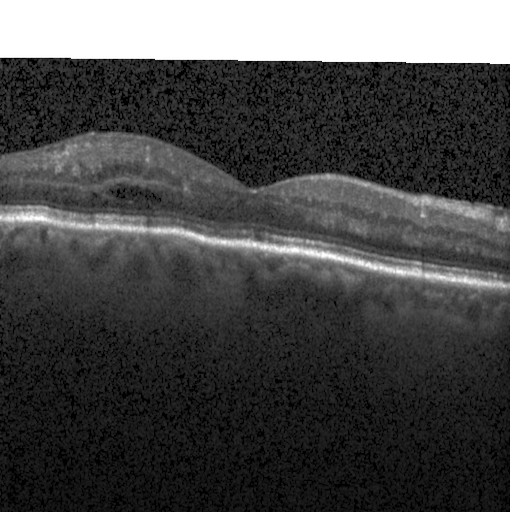
Optical coherence tomography B-scan. Finding: diabetic macular edema.